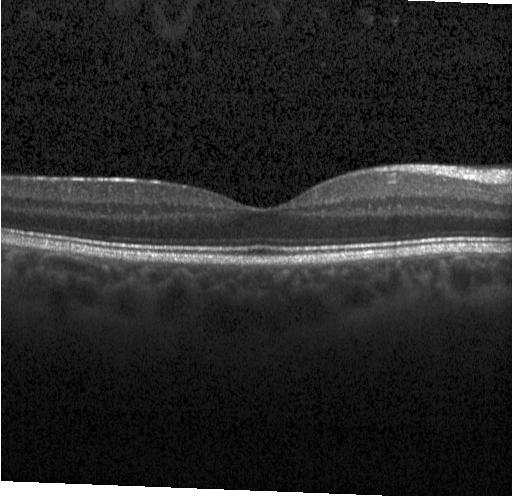

Acquired on a Heidelberg Spectralis; SD-OCT; retinal OCT cross-section; through the macula — Assessment: no choroidal neovascularization, diabetic macular edema, or drusen.